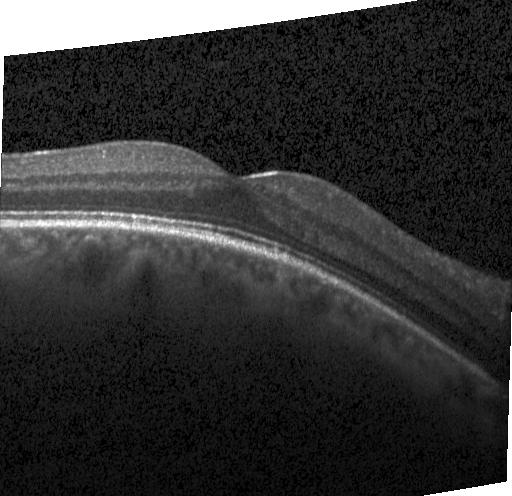
Impression: no choroidal neovascularization, diabetic macular edema, or drusen.